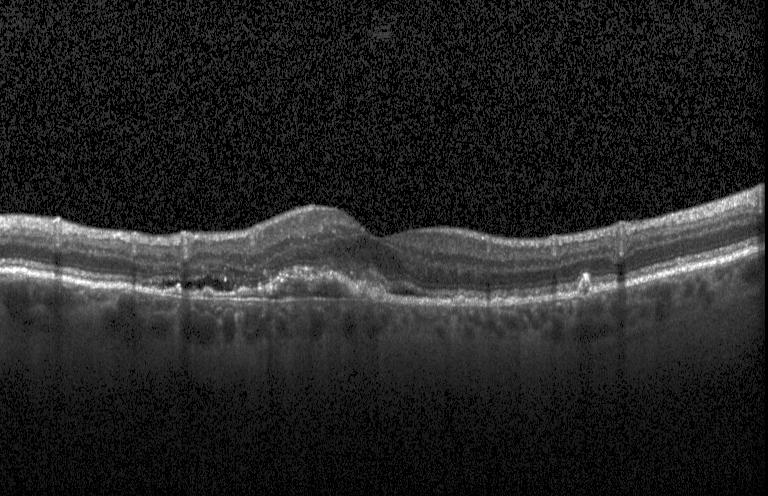
Retinal OCT cross-section. OCT finding: a choroidal neovascular membrane.